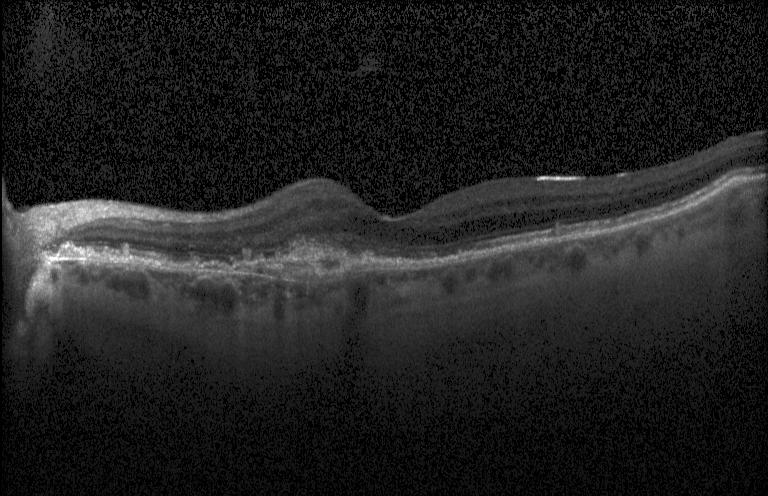
OCT scan showing CNV.